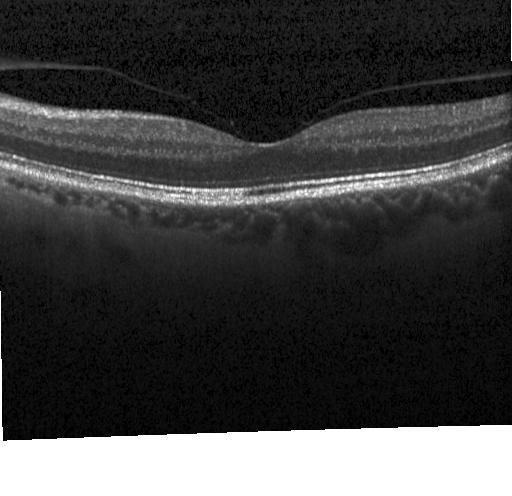 Macular scan; spectral-domain OCT; Heidelberg Spectralis OCT system; retinal OCT cross-section. Finding: neither choroidal neovascularization, diabetic macular edema, nor drusen.